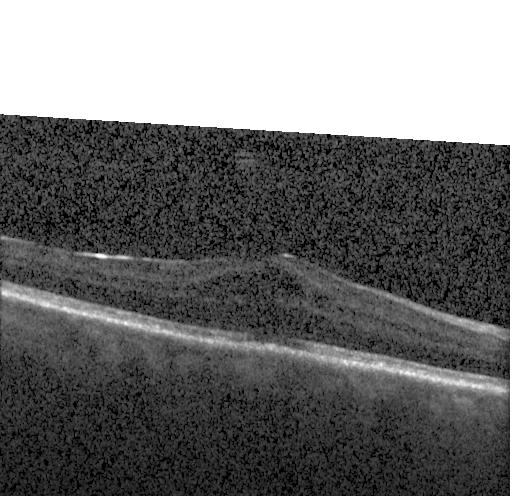
Retinal OCT cross-section.
Diagnosis: diabetic macular edema (DME).